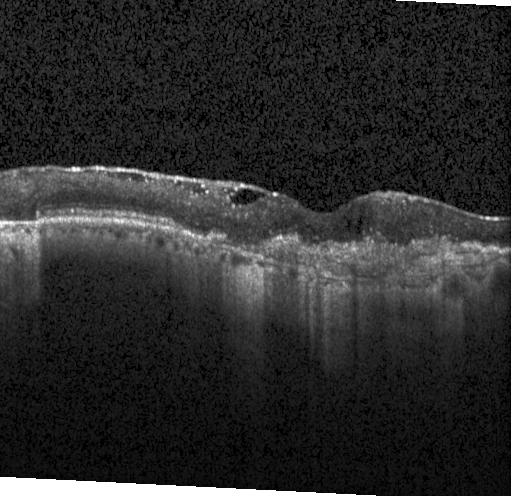 Optical coherence tomography B-scan — Impression: a choroidal neovascular membrane.